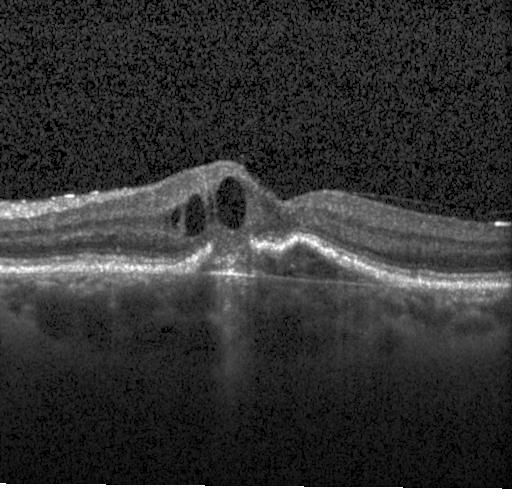 Retinal OCT cross-section. Diagnosis: a choroidal neovascular membrane.